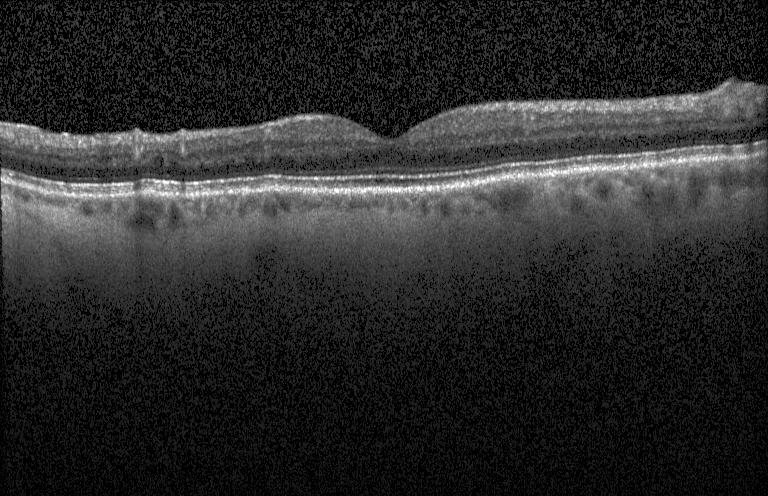

Optical coherence tomography scan · spectral-domain optical coherence tomography — Assessment: no choroidal neovascularization, diabetic macular edema, or drusen.